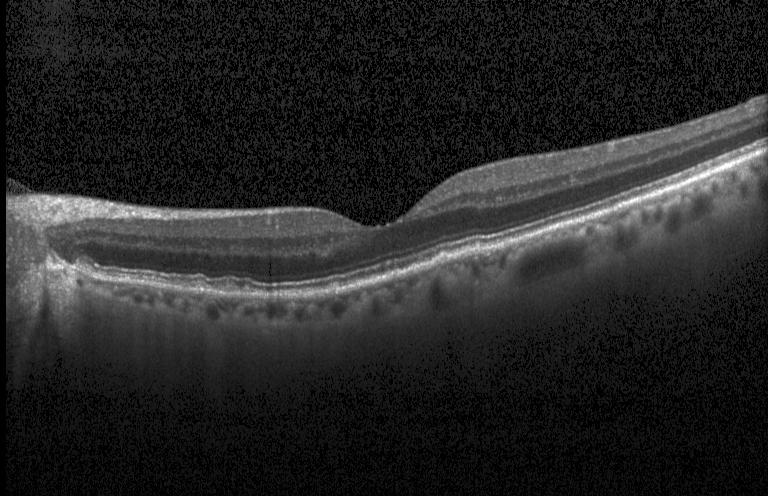

Through the macula. Instrument: Heidelberg Spectralis. OCT line scan — Macular OCT: drusen.